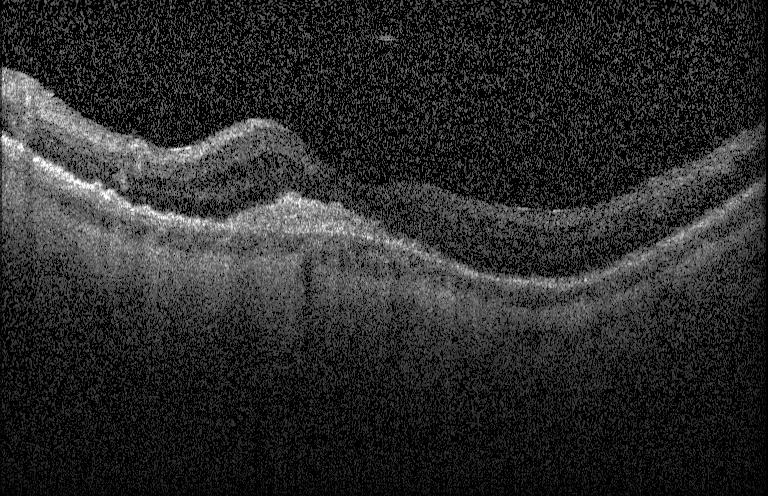
Retinal OCT cross-section showing a choroidal neovascular membrane.